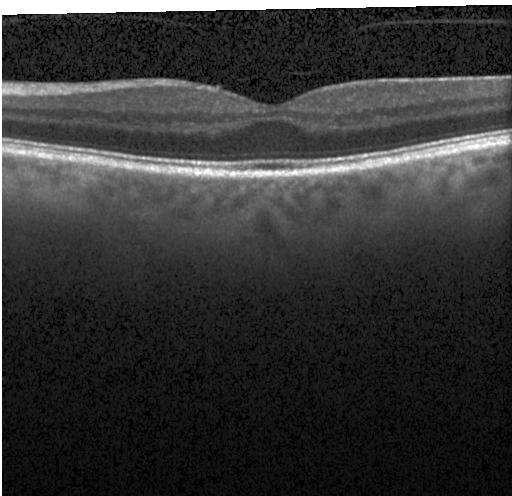

Through the macula. Retinal OCT B-scan. This B-scan demonstrates no evidence of choroidal neovascularization, diabetic macular edema, or drusen.